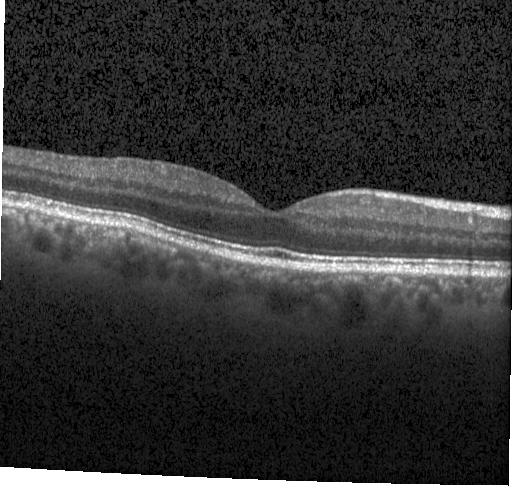

Acquired on a Heidelberg Spectralis. Retinal OCT B-scan. Through the macula. Spectral-domain OCT.
This B-scan demonstrates neither choroidal neovascularization, diabetic macular edema, nor drusen.